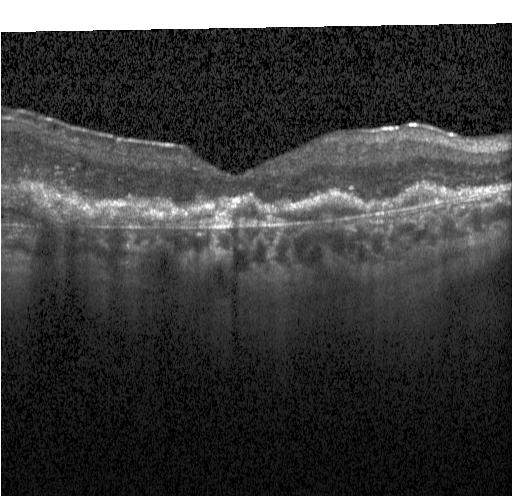 Diagnosis: a choroidal neovascular membrane.